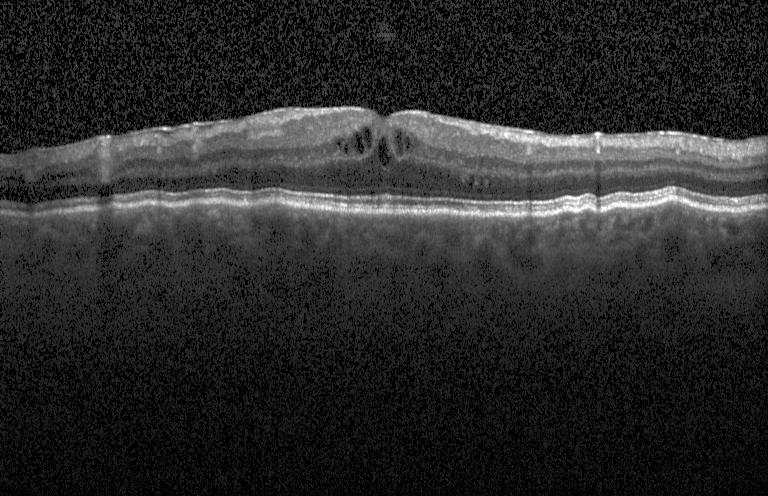 OCT B-scan. SD-OCT. Instrument: Heidelberg Spectralis. Through the macula.
DME.